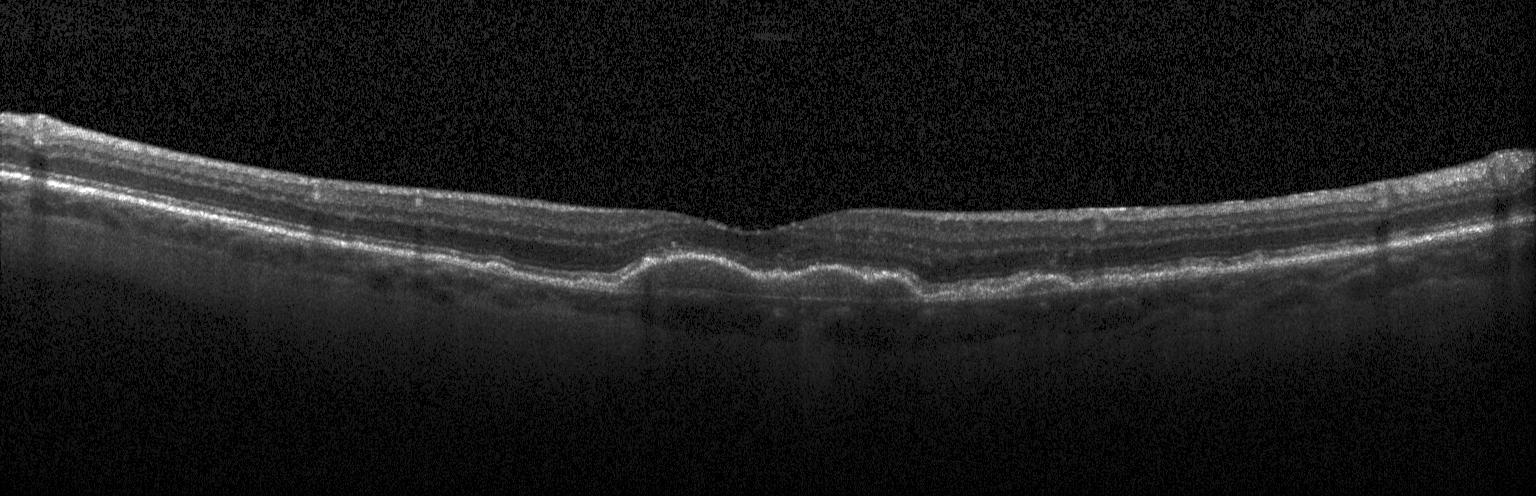
Optical coherence tomography scan.
Diagnosis: a choroidal neovascular membrane.